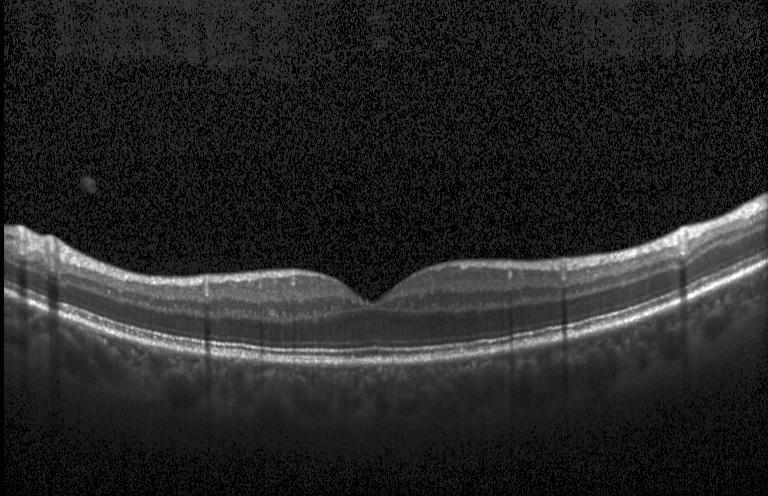 Optical coherence tomography B-scan.
Finding: no CNV, no DME, and no drusen.